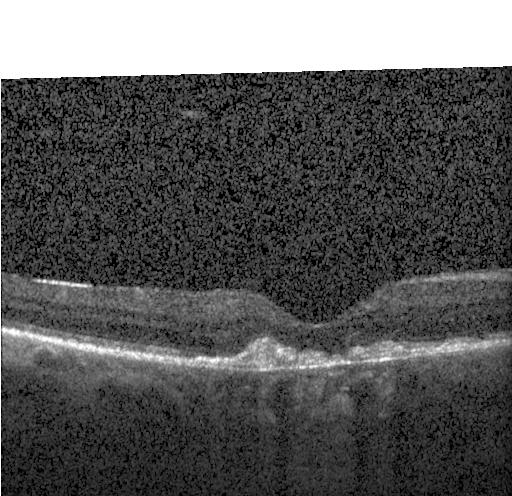
Horizontal scan through the fovea. Retinal OCT B-scan. Dx: a choroidal neovascular membrane.